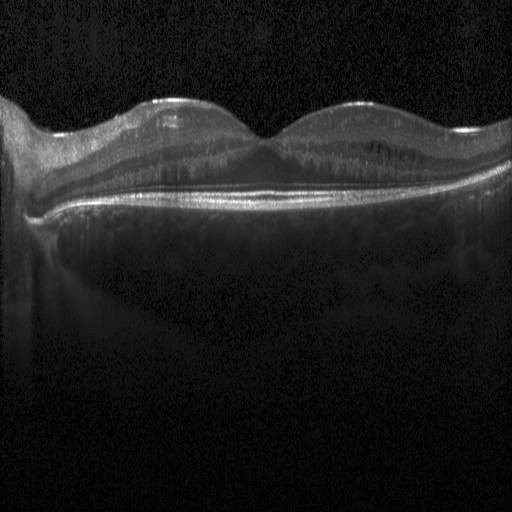 DME.